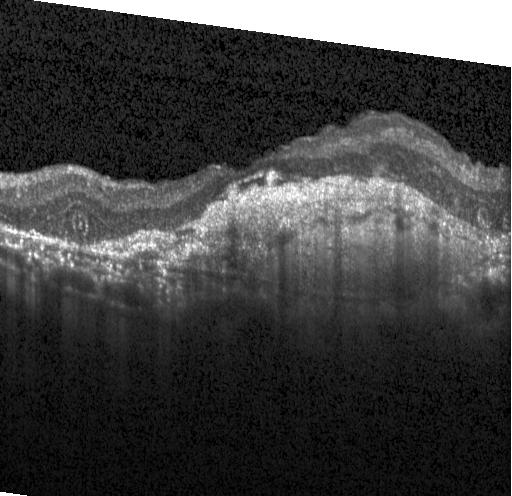
Diagnosis: a choroidal neovascular membrane.